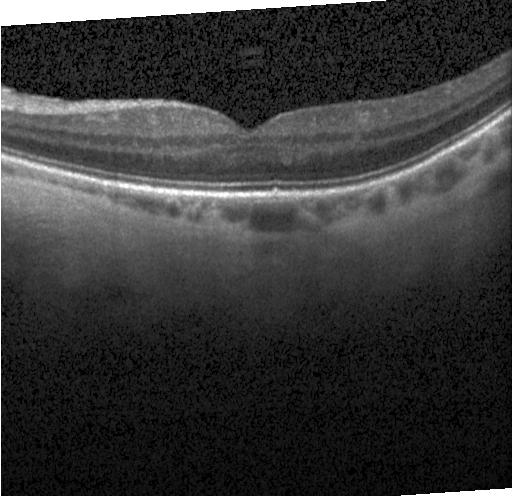 Dx: drusen.